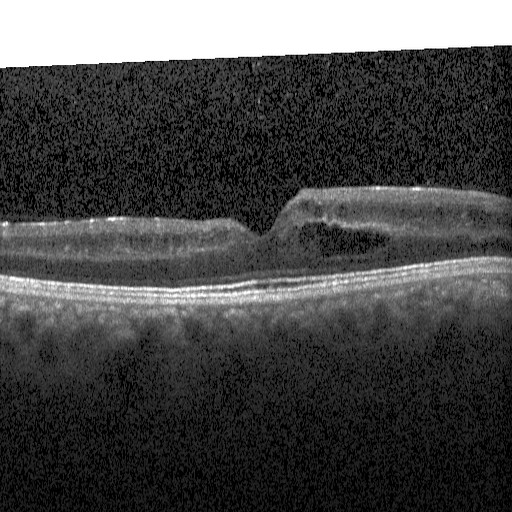
Retinal OCT cross-section. Through the macula. SD-OCT
Finding: DME.